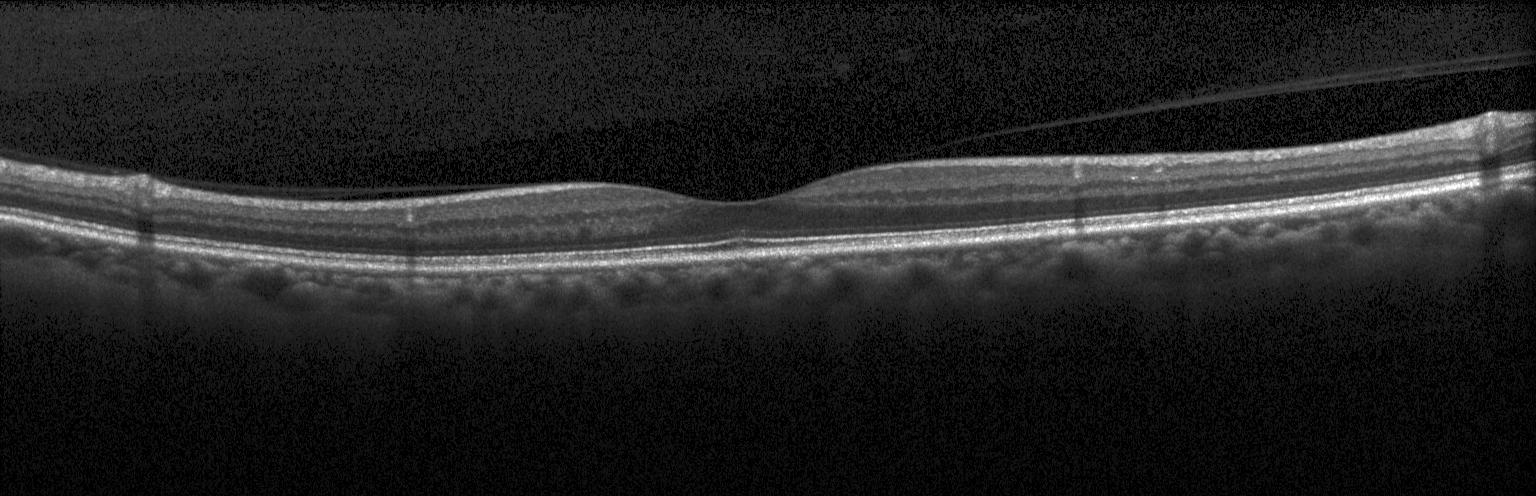

Diagnosis: no CNV, DME, or drusen.